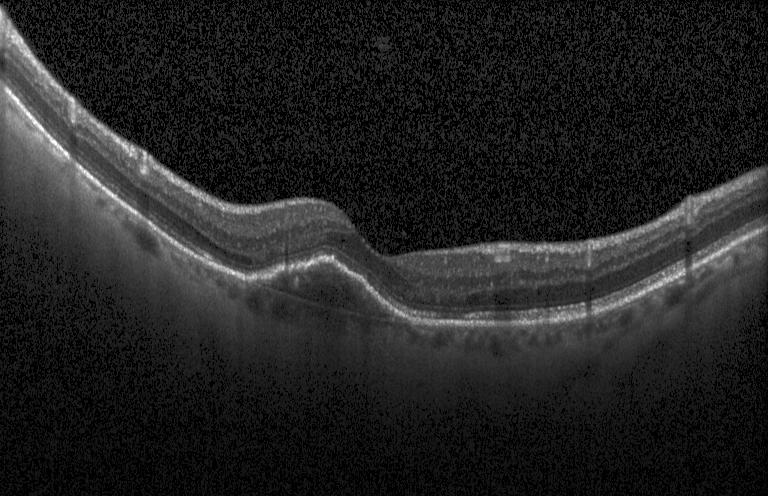 Finding: a choroidal neovascular membrane.